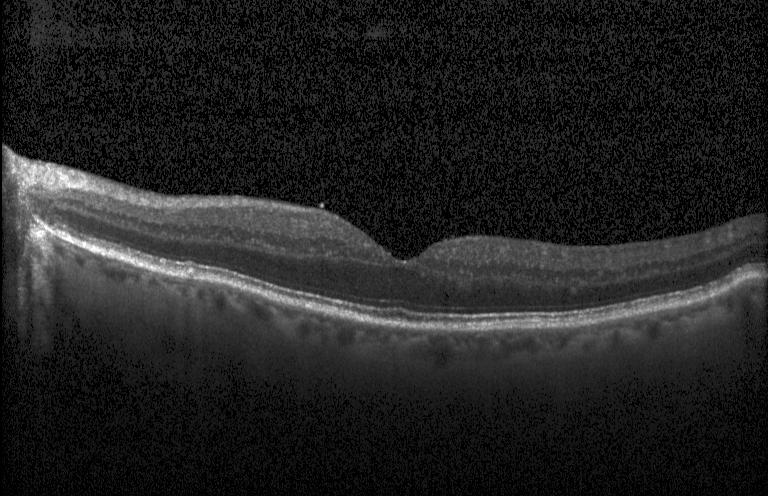

Dx: no evidence of choroidal neovascularization, diabetic macular edema, or drusen.